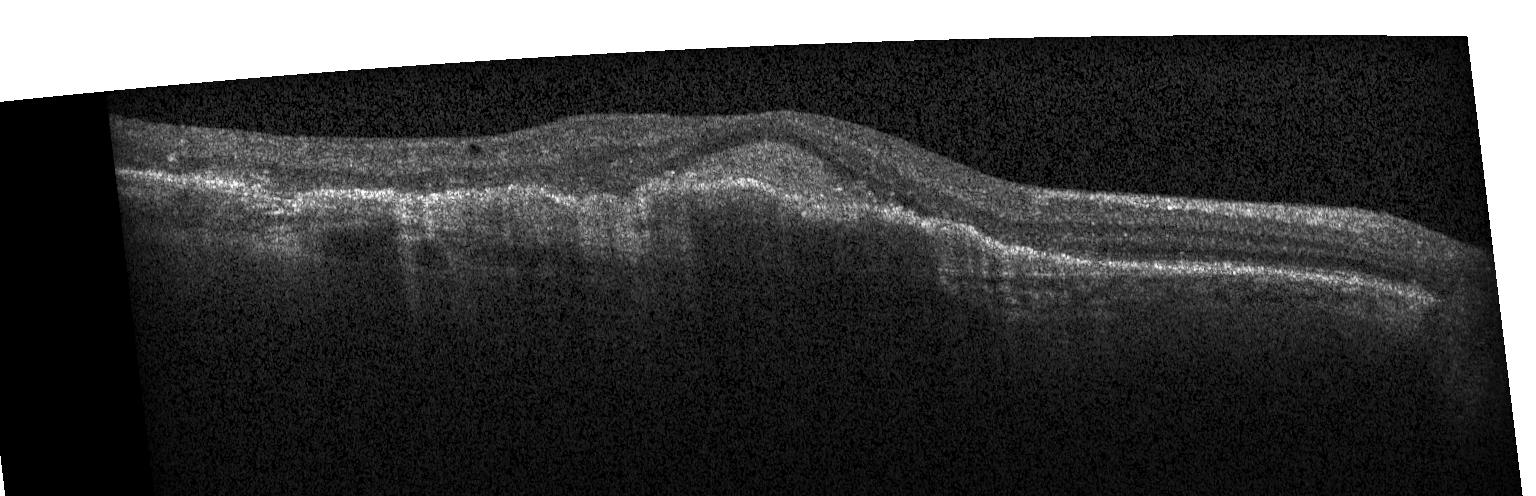

Retinal OCT B-scan. SD-OCT. Heidelberg Spectralis — This B-scan demonstrates a choroidal neovascular membrane.